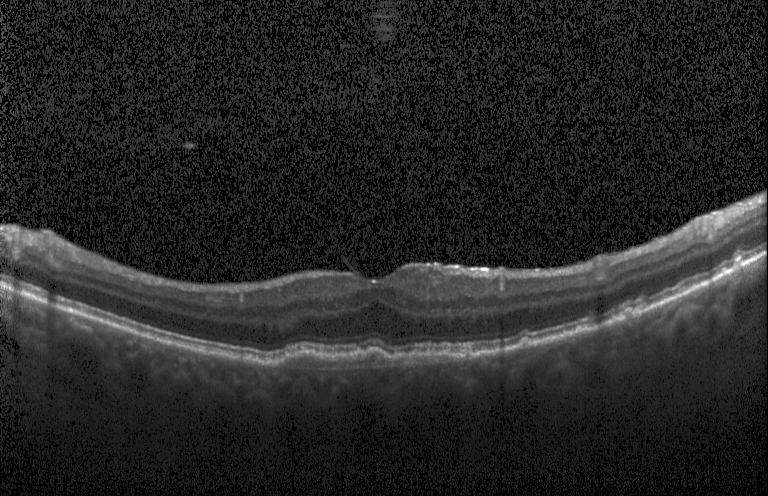

Spectral-domain OCT B-scan: a choroidal neovascular membrane.